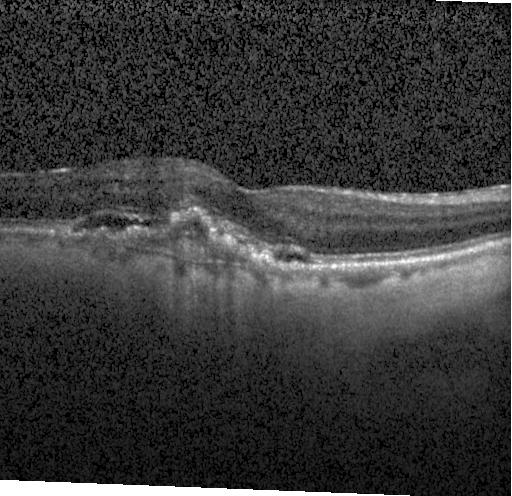 Retinal OCT B-scan · spectral-domain optical coherence tomography · fovea-centered. Impression: a choroidal neovascular membrane.